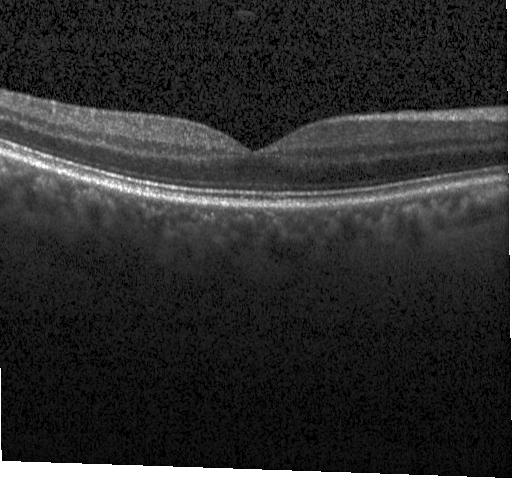

Diagnosis: neither CNV, DME, nor drusen.